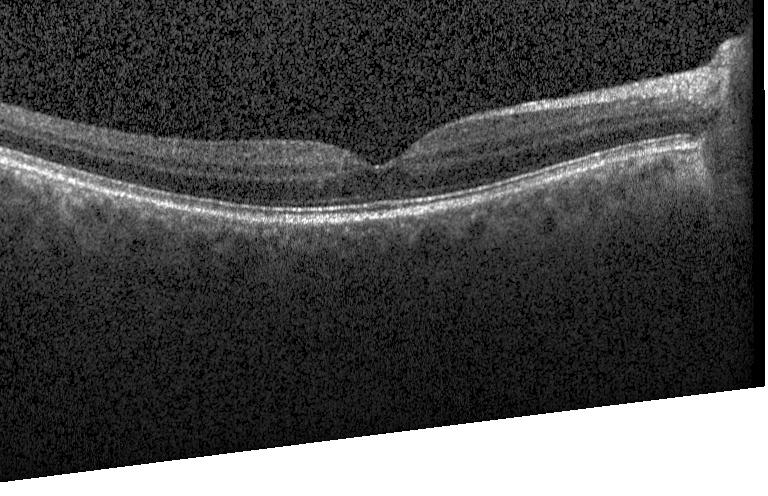 Horizontal scan through the fovea; spectral-domain OCT; OCT B-scan; Heidelberg Spectralis. Diagnosis: no evidence of choroidal neovascularization, diabetic macular edema, or drusen.